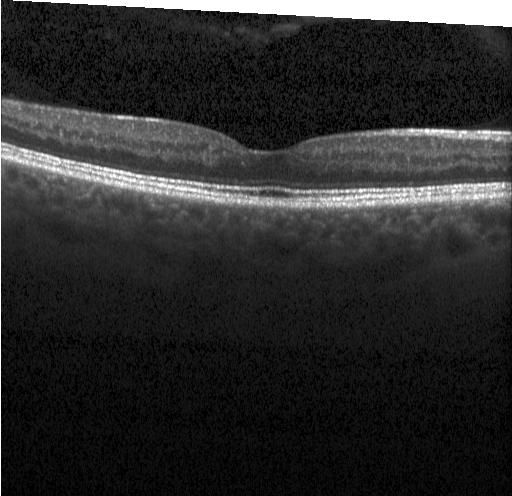
Heidelberg Spectralis OCT system. Spectral-domain OCT. OCT line scan. Macular scan — Diagnosis: no choroidal neovascularization, diabetic macular edema, or drusen.